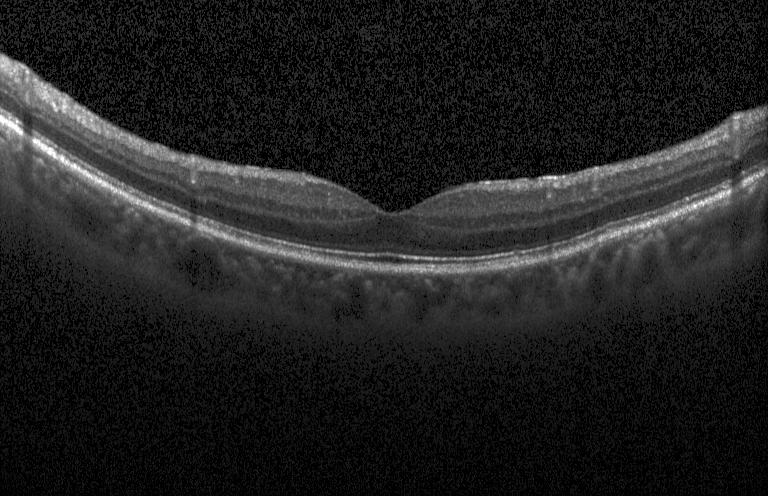
Spectral-domain optical coherence tomography; Heidelberg Spectralis OCT system; retinal OCT B-scan.
Finding: no evidence of choroidal neovascularization, diabetic macular edema, or drusen.